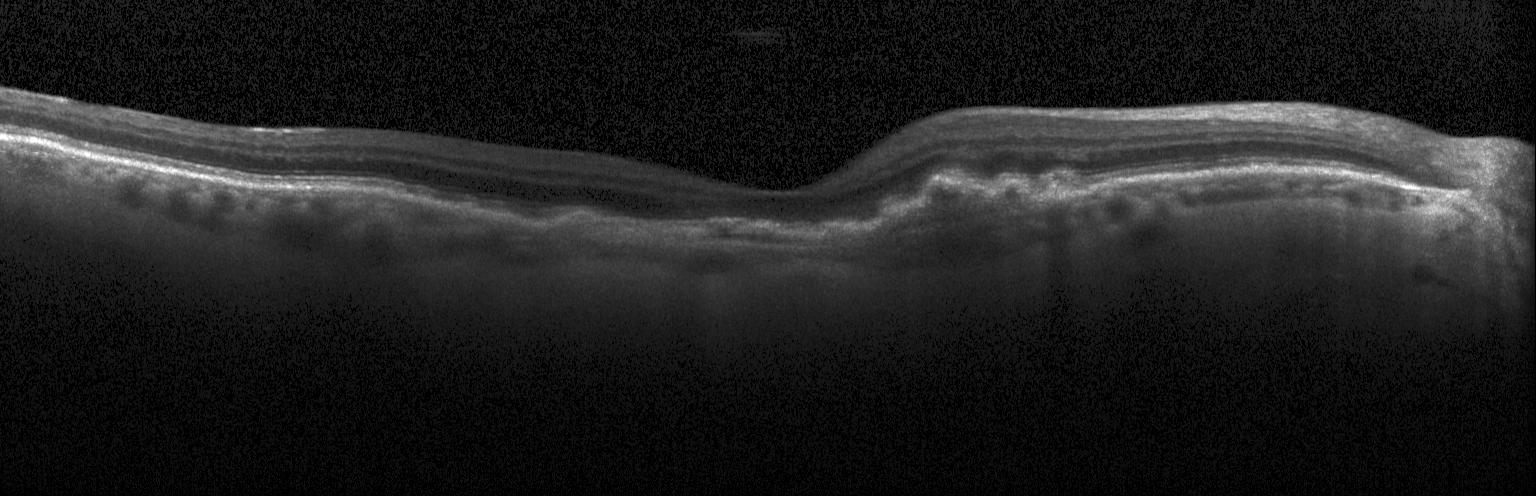

Impression: a choroidal neovascular membrane.